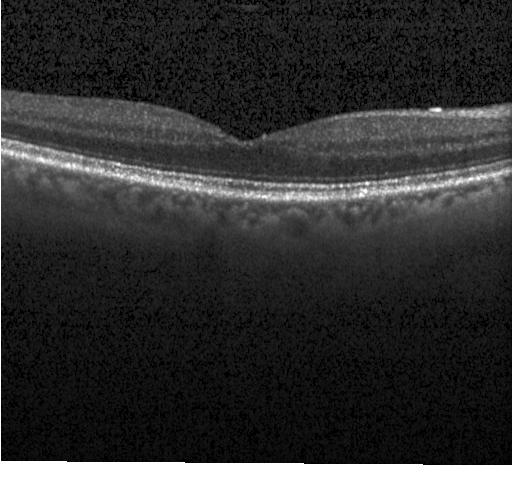 Macular OCT demonstrating no evidence of CNV, DME, or drusen.